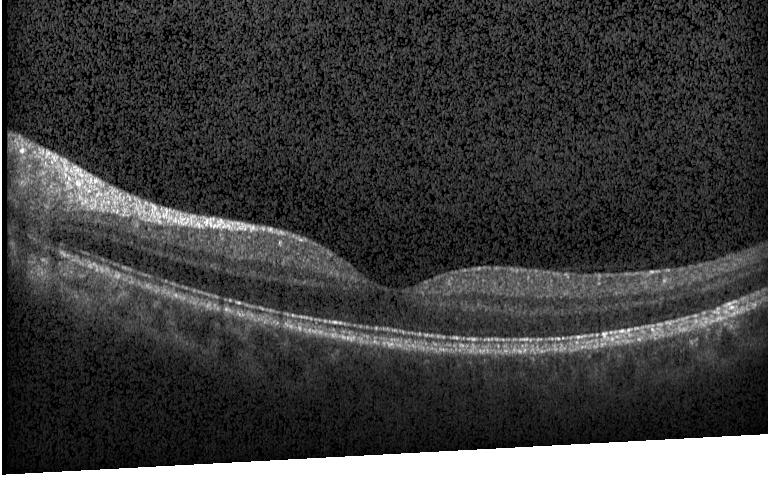
Acquired on a Heidelberg Spectralis · spectral-domain optical coherence tomography · optical coherence tomography scan
Dx: no choroidal neovascularization, no diabetic macular edema, and no drusen.